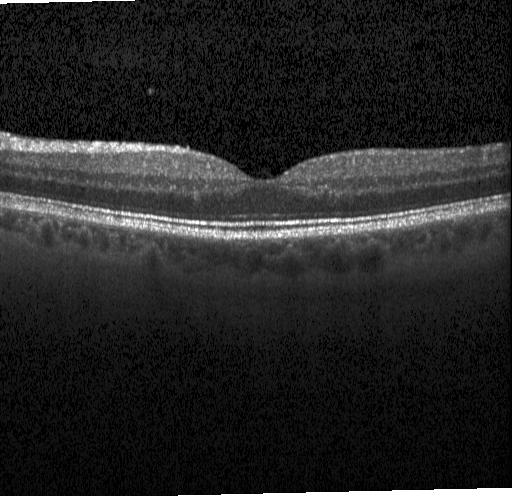

Retinal OCT B-scan. Macular scan.
Finding: neither CNV, DME, nor drusen.